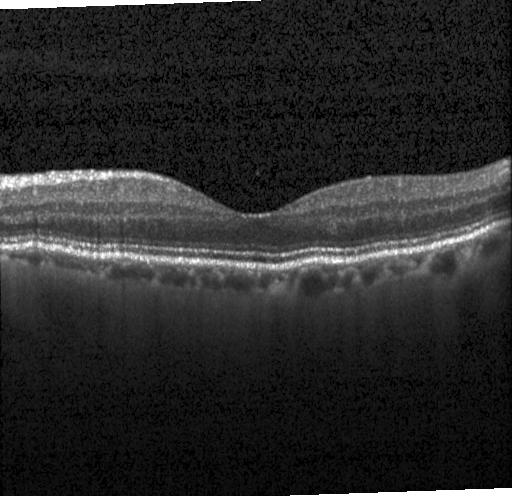
OCT line scan; centered on the fovea — Impression: no choroidal neovascularization, diabetic macular edema, or drusen.